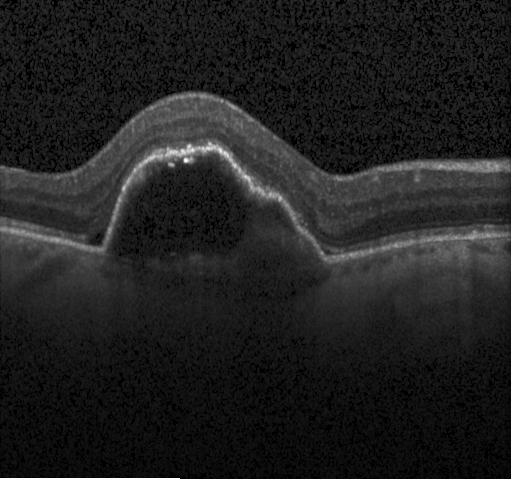
Fovea-centered. OCT B-scan. Impression: a choroidal neovascular membrane.